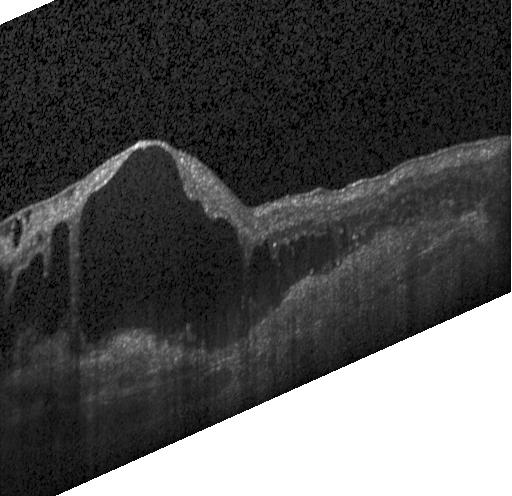

Dx: choroidal neovascularization.